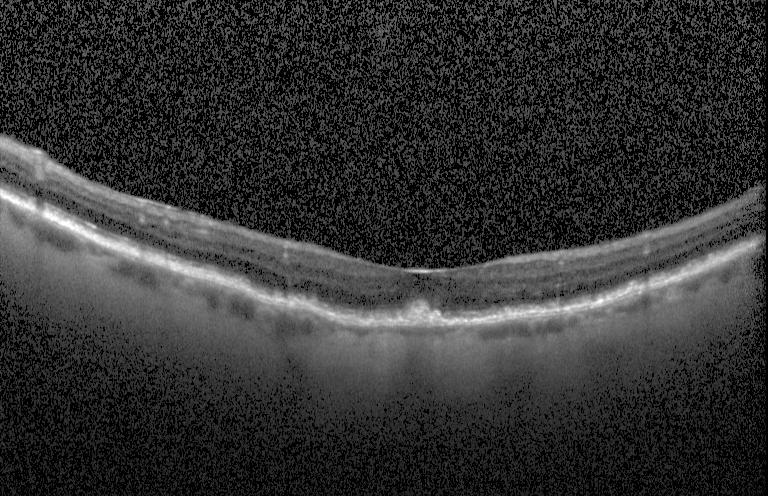 Macular OCT demonstrating a choroidal neovascular membrane.